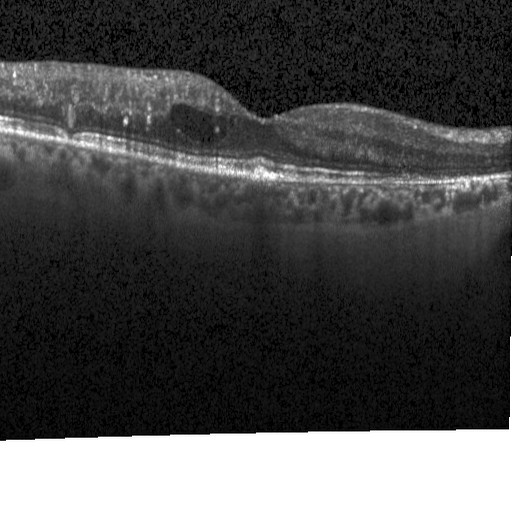

The scan shows diabetic macular edema.